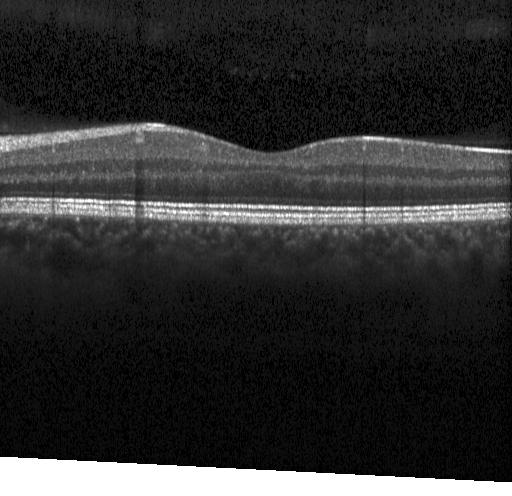 Optical coherence tomography scan — Dx: no choroidal neovascularization, no diabetic macular edema, and no drusen.